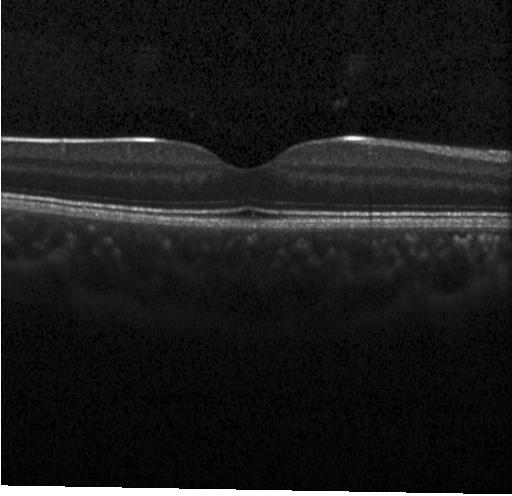

Retinal OCT cross-section. No evidence of CNV, DME, or drusen.